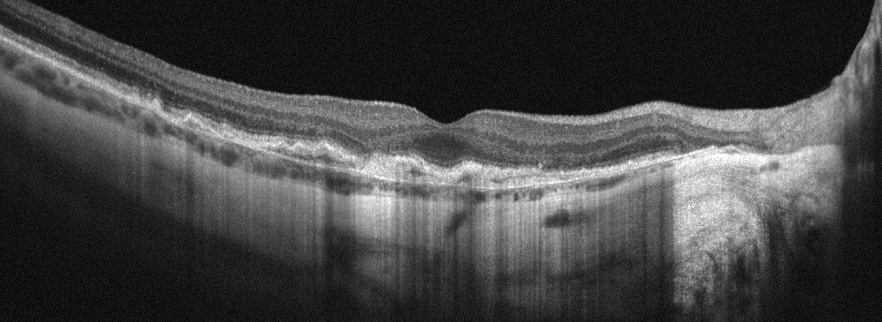
AMD.